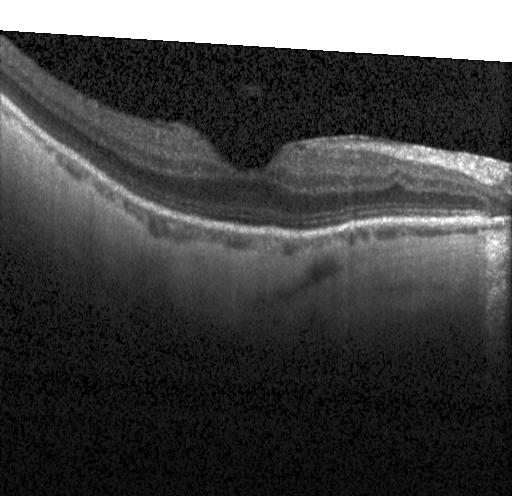
Optical coherence tomography B-scan. Horizontal scan through the fovea — Finding: no CNV, no DME, and no drusen.